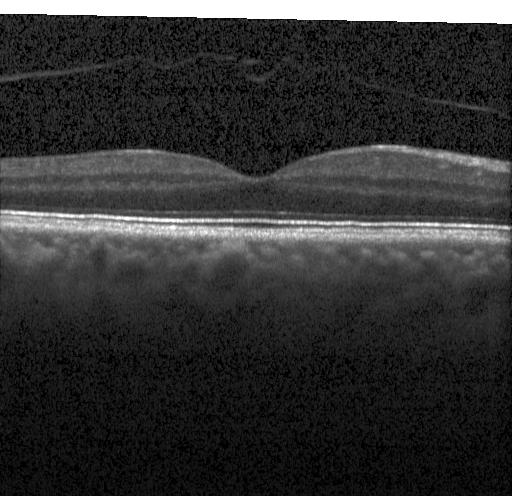 Macular OCT: no evidence of CNV, DME, or drusen.